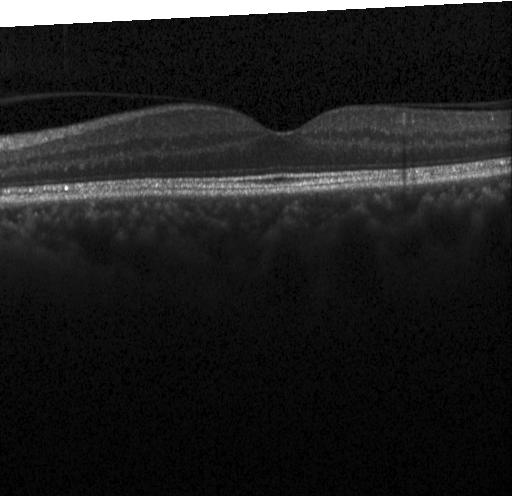 No CNV, DME, or drusen.